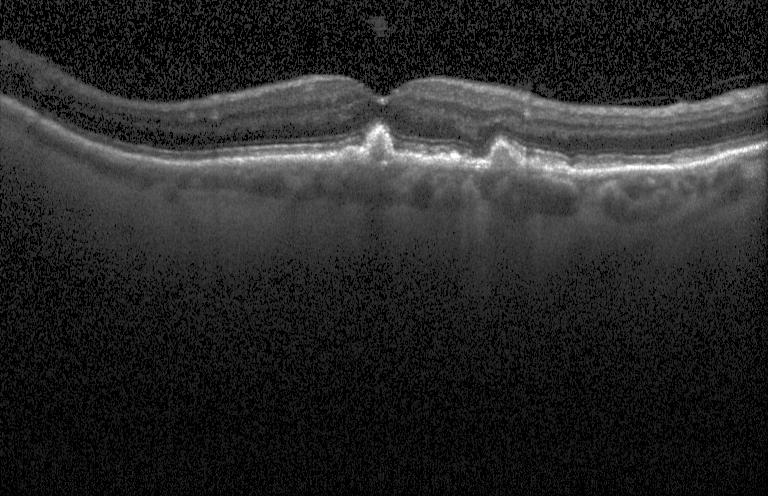 Retinal OCT B-scan. Diagnosis: drusen.